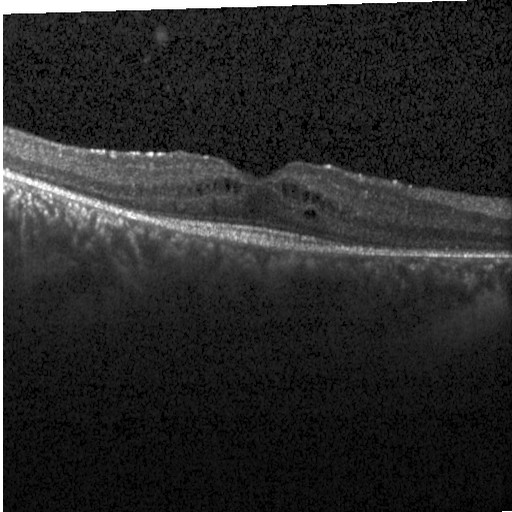

OCT B-scan. The scan shows diabetic macular edema (DME).